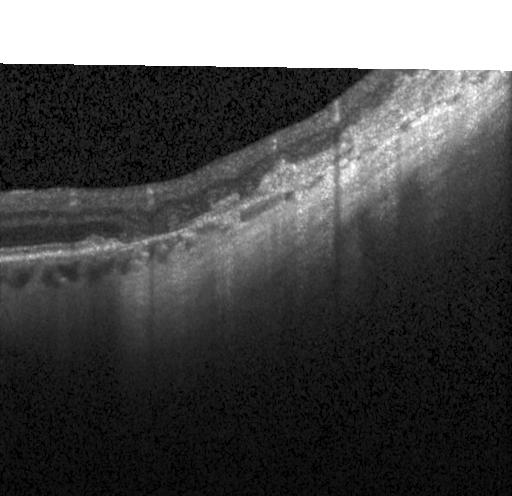 Dx: a choroidal neovascular membrane.